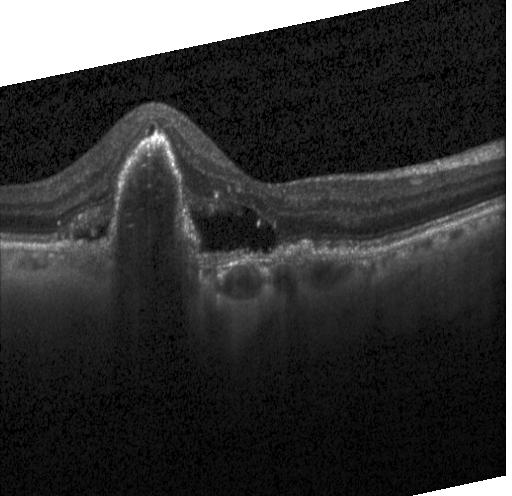 Optical coherence tomography scan; spectral-domain OCT; horizontal scan through the fovea; Heidelberg Spectralis.
The scan shows choroidal neovascularization (CNV).